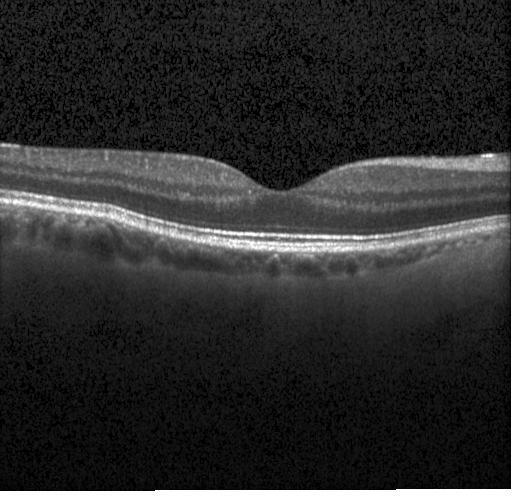 Horizontal scan through the fovea; optical coherence tomography B-scan; spectral-domain OCT; instrument: Heidelberg Spectralis
OCT finding: neither choroidal neovascularization, diabetic macular edema, nor drusen.